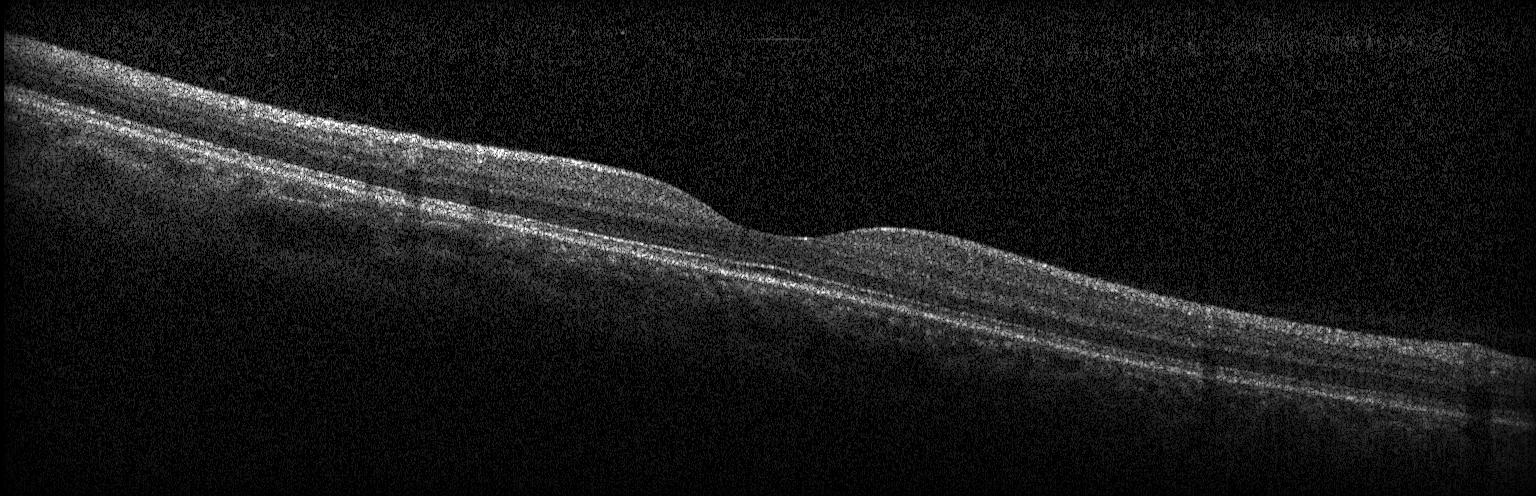 Optical coherence tomography scan. Spectral-domain optical coherence tomography. Heidelberg Spectralis. Impression: no evidence of choroidal neovascularization, diabetic macular edema, or drusen.